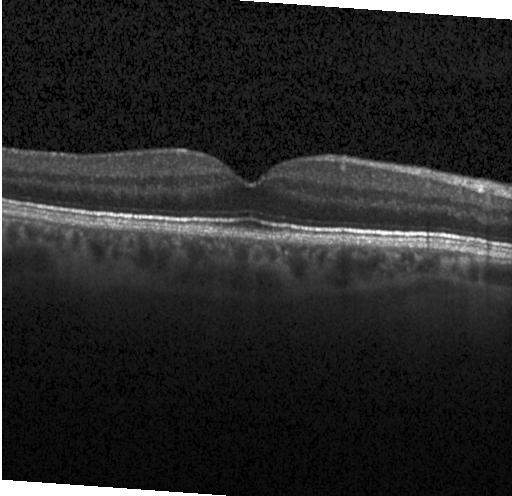
Spectral-domain optical coherence tomography · macular scan · retinal OCT cross-section
Dx: neither choroidal neovascularization, diabetic macular edema, nor drusen.